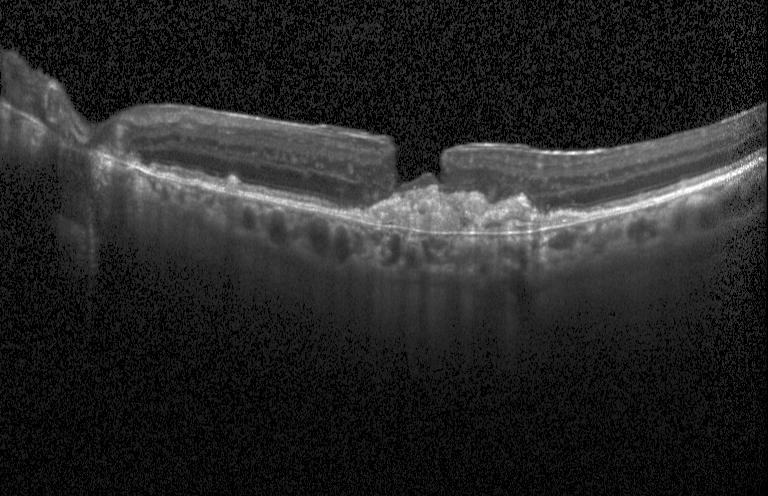

Through the macula, OCT line scan, Heidelberg Spectralis OCT system, spectral-domain optical coherence tomography. Impression: choroidal neovascularization (CNV).